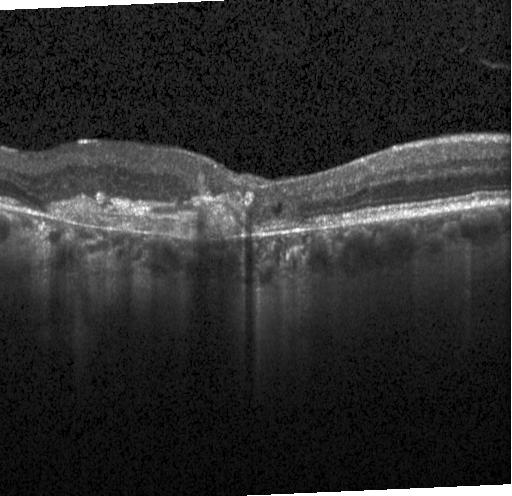 Macular scan · SD-OCT · retinal OCT B-scan.
Diagnosis: a choroidal neovascular membrane.